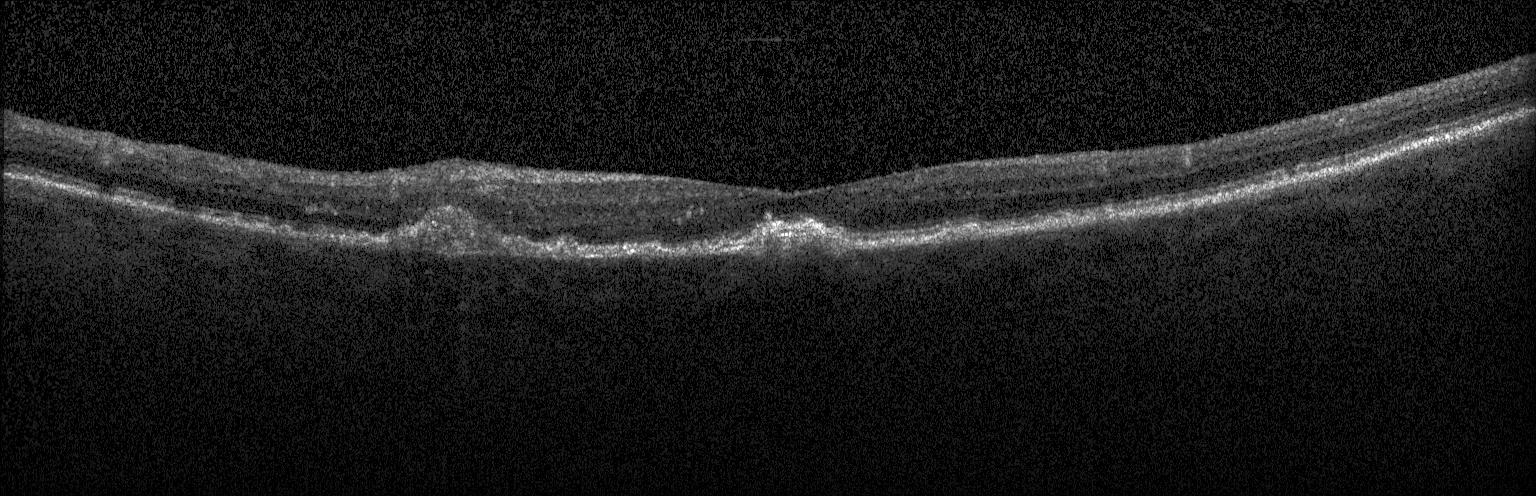 OCT scan showing choroidal neovascularization.